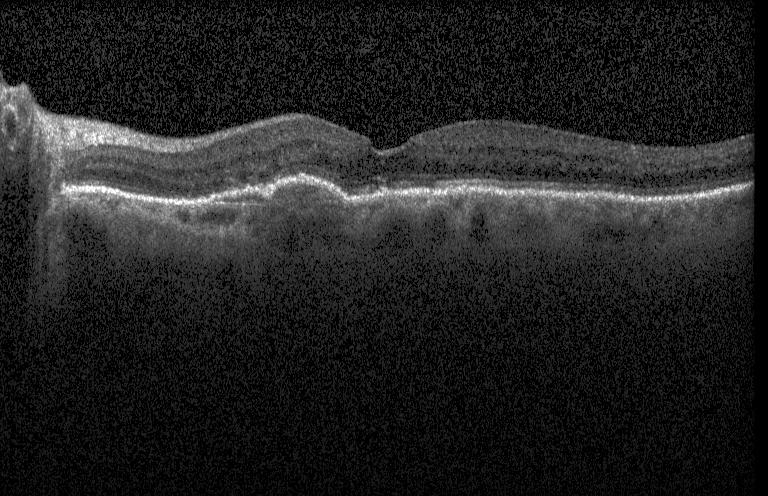 Optical coherence tomography scan
Assessment: a choroidal neovascular membrane.